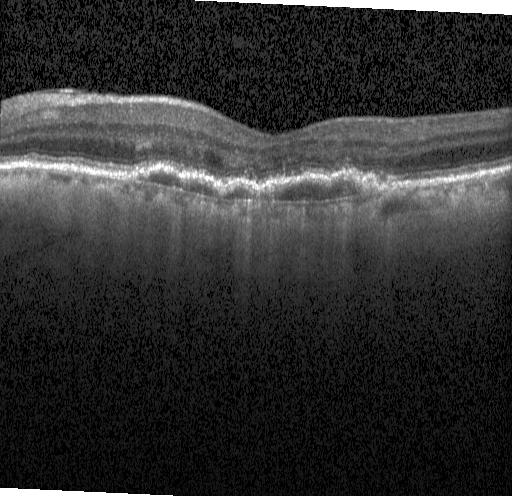

Optical coherence tomography scan, spectral-domain OCT. CNV.